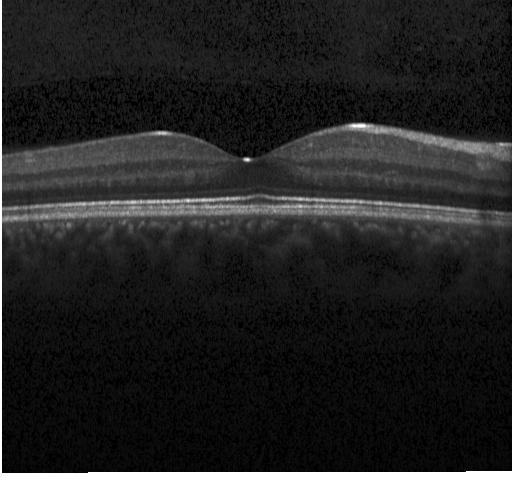
Impression: no choroidal neovascularization, diabetic macular edema, or drusen.